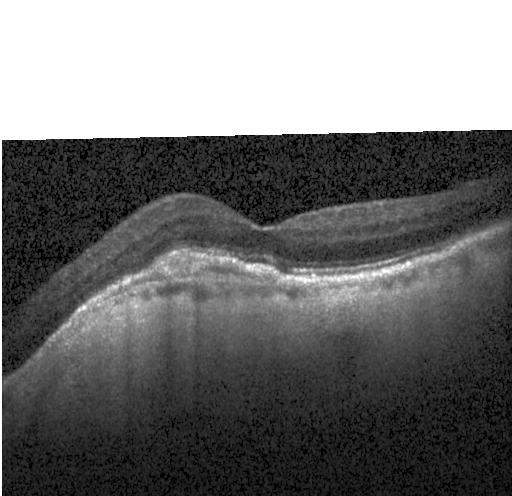
Instrument: Heidelberg Spectralis. Spectral-domain OCT. Optical coherence tomography B-scan. Macular scan — Finding: choroidal neovascularization (CNV).